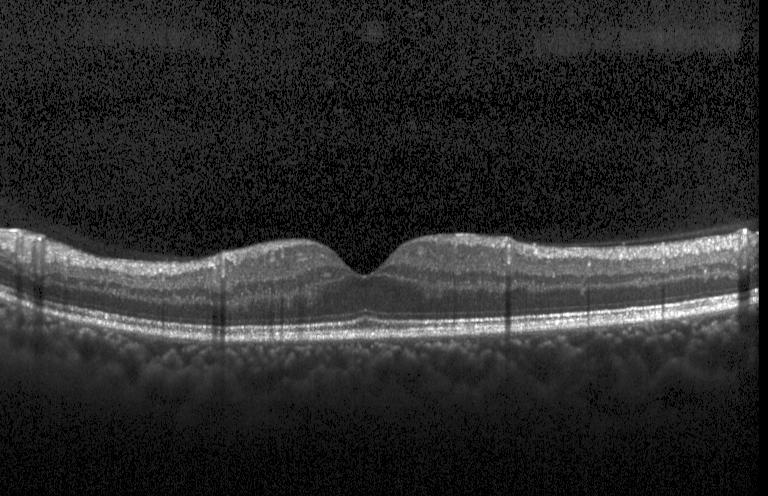 Heidelberg Spectralis OCT system, OCT B-scan
No evidence of choroidal neovascularization, diabetic macular edema, or drusen.